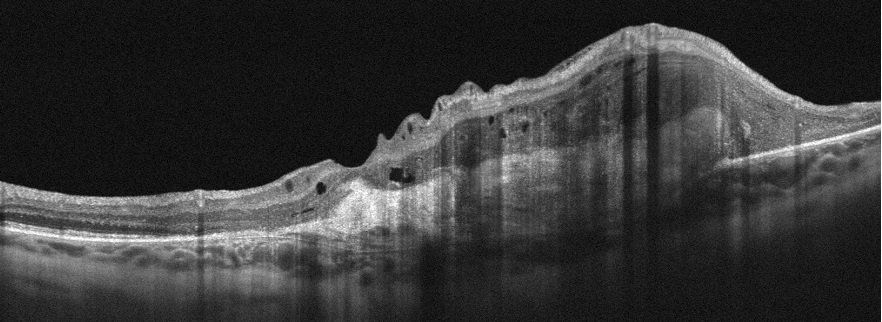
Macular scan. OCT line scan.
Impression: age-related macular degeneration.